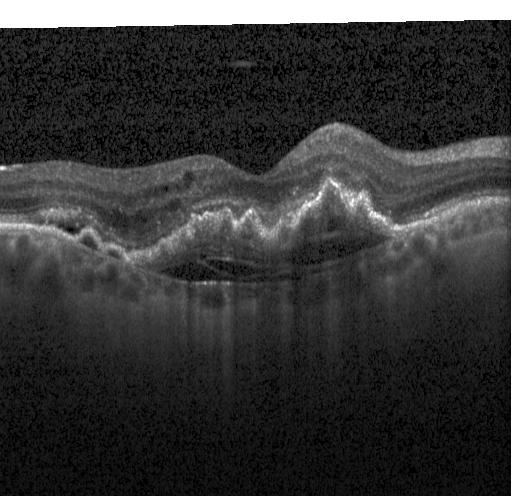 Retinal OCT cross-section
Diagnosis: choroidal neovascularization.